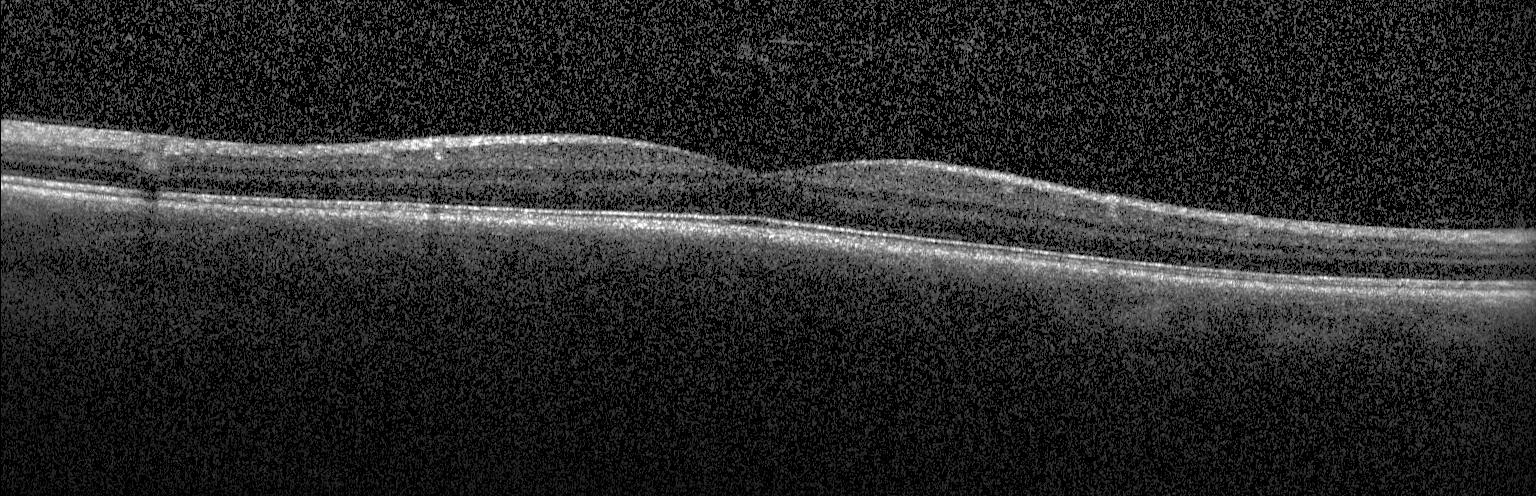
Retinal OCT B-scan.
No evidence of CNV, DME, or drusen.